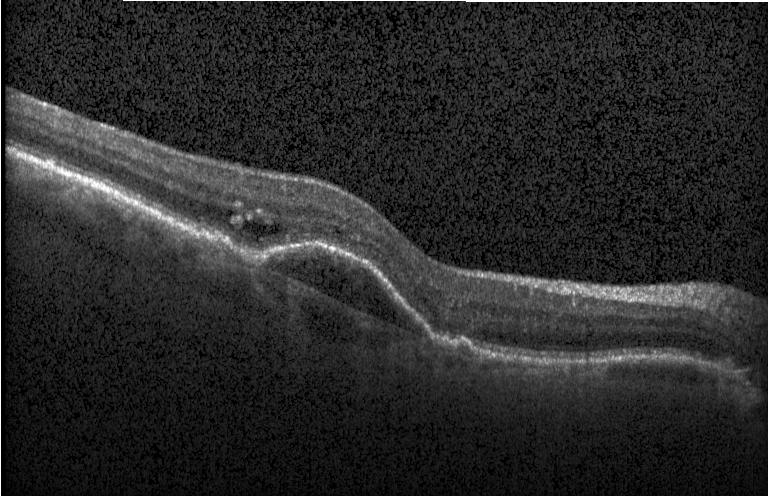

Finding: choroidal neovascularization (CNV).